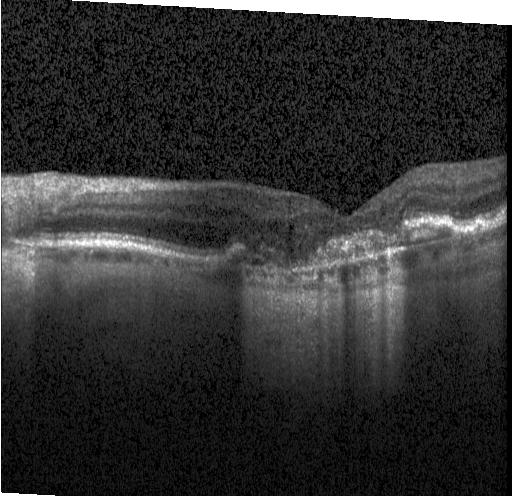 Optical coherence tomography B-scan · Heidelberg Spectralis OCT system · spectral-domain OCT
Macular OCT: CNV.